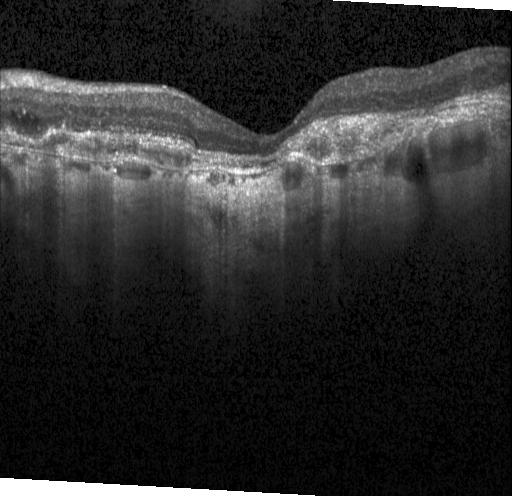 OCT finding: a choroidal neovascular membrane.